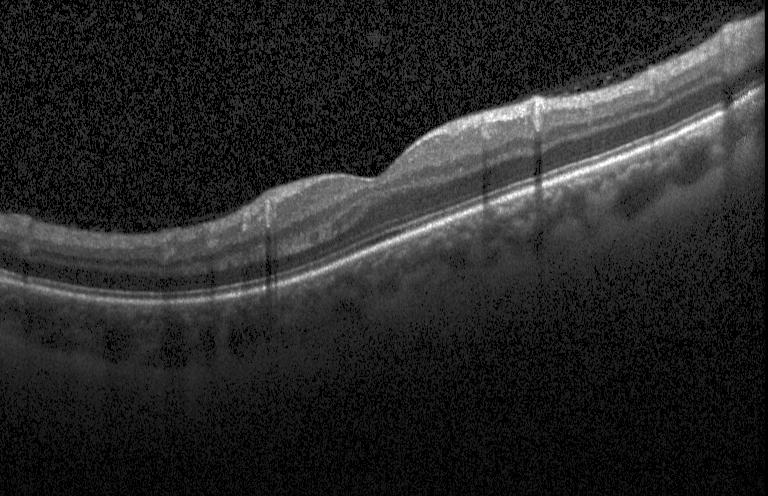
Horizontal scan through the fovea · optical coherence tomography scan.
Impression: no choroidal neovascularization, no diabetic macular edema, and no drusen.